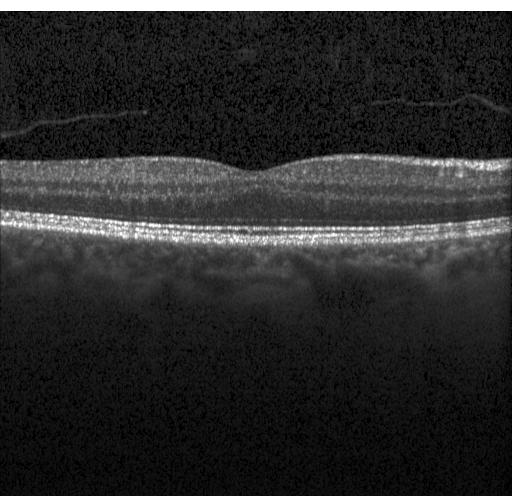 Dx: no CNV, no DME, and no drusen.